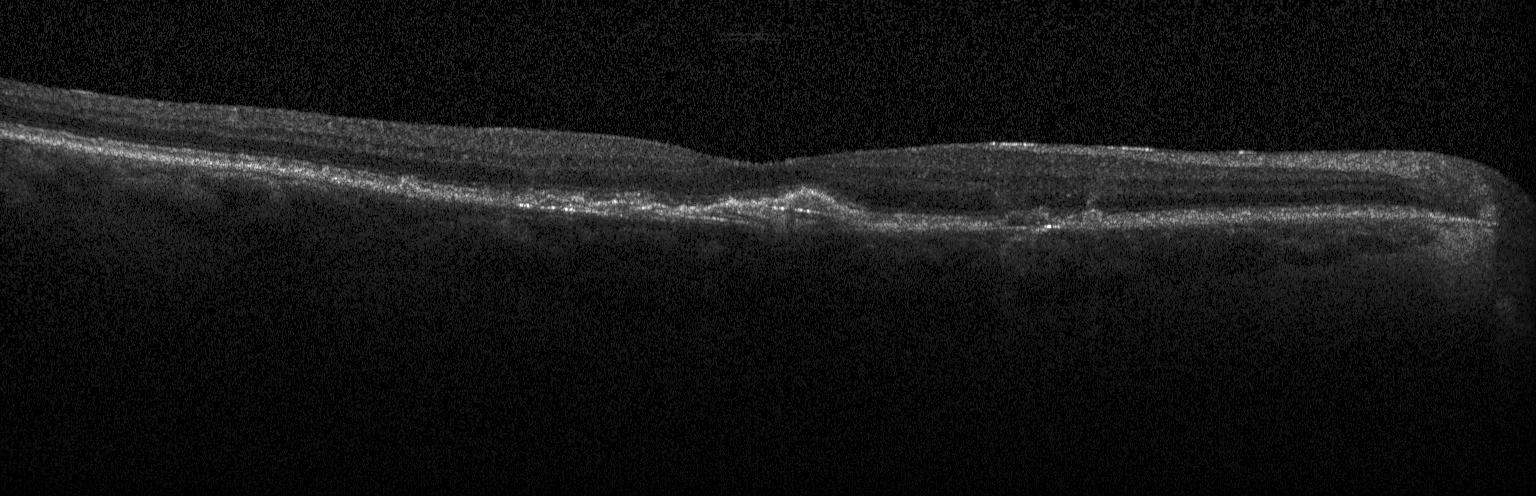

OCT B-scan.
Dx: CNV.